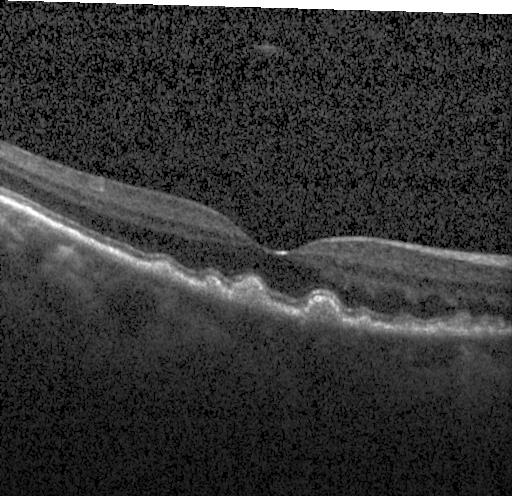

Retinal OCT B-scan. Heidelberg Spectralis OCT system. Spectral-domain optical coherence tomography. Sub-RPE drusenoid deposits.